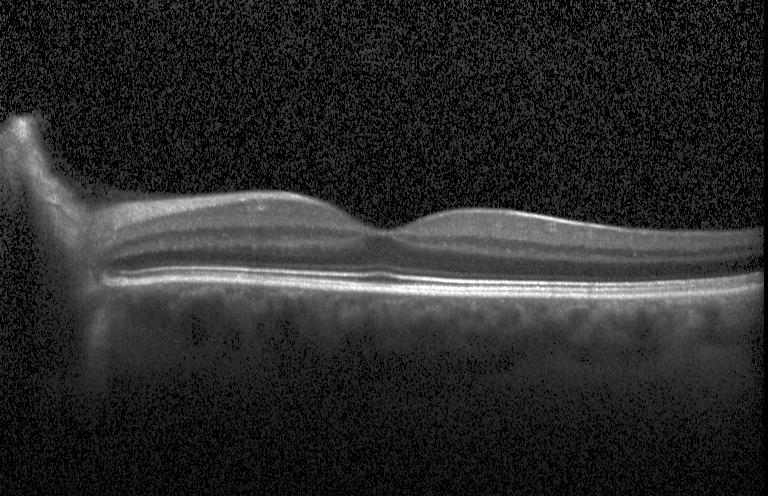
Spectral-domain optical coherence tomography, instrument: Heidelberg Spectralis, optical coherence tomography B-scan, fovea-centered.
The scan shows neither choroidal neovascularization, diabetic macular edema, nor drusen.